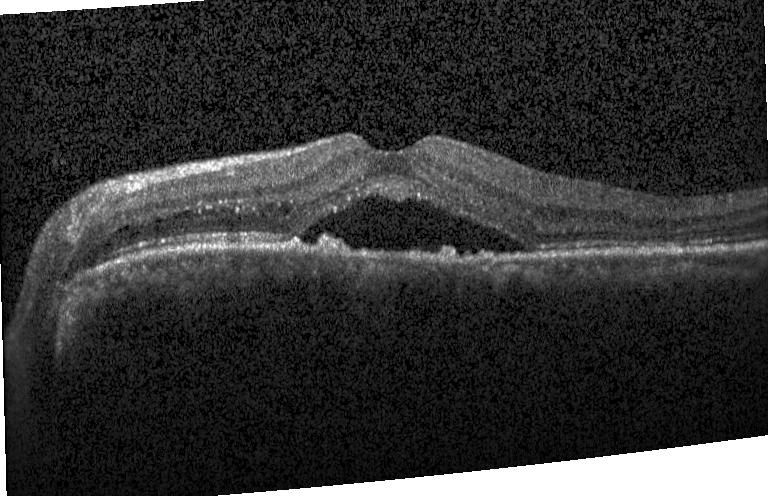 Optical coherence tomography scan.
This B-scan demonstrates a choroidal neovascular membrane.